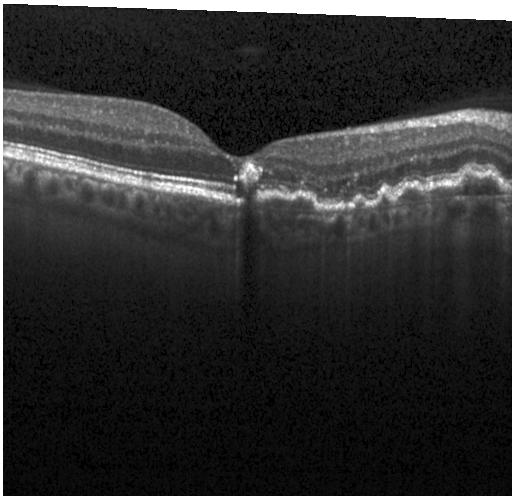
Diagnosis: CNV.